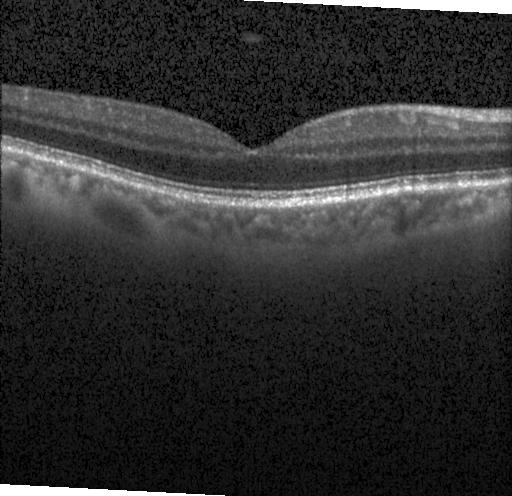
This B-scan demonstrates no evidence of CNV, DME, or drusen.